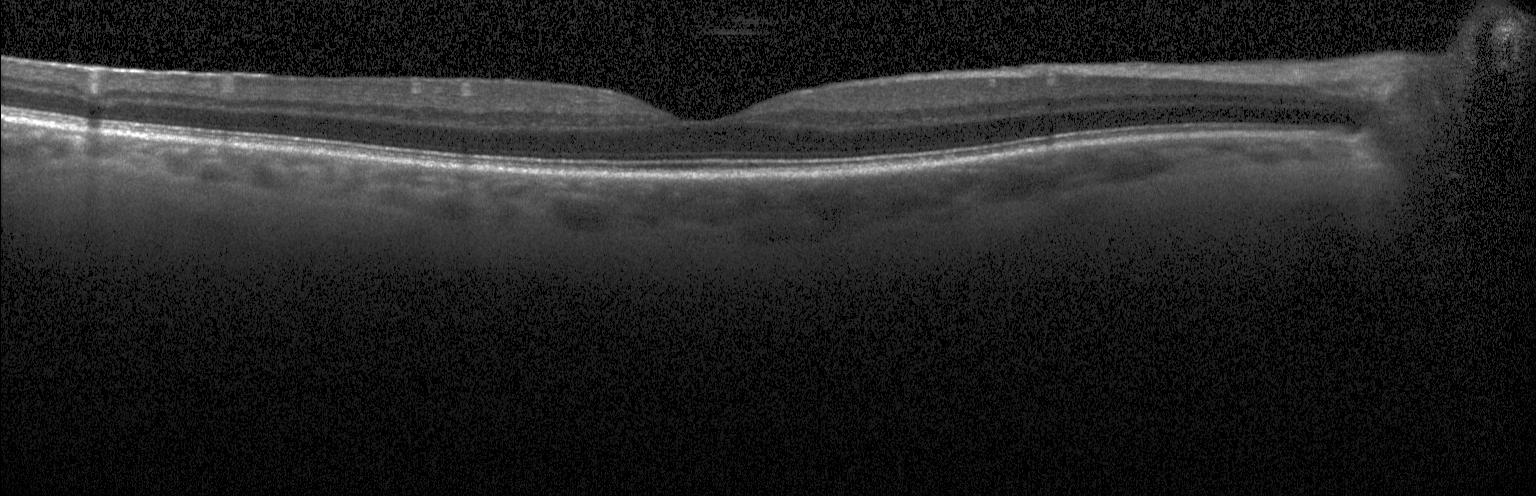 Heidelberg Spectralis OCT system; retinal OCT B-scan; macular scan; spectral-domain OCT. OCT finding: no evidence of CNV, DME, or drusen.